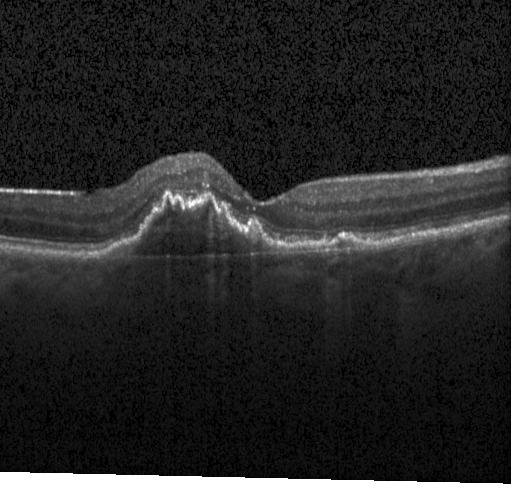 Horizontal scan through the fovea · OCT line scan.
Finding: a choroidal neovascular membrane.